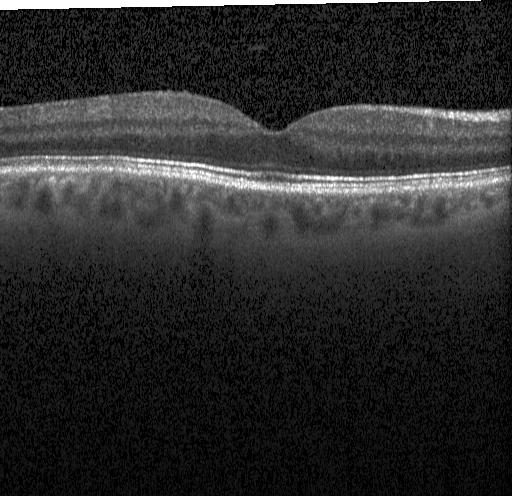

Horizontal scan through the fovea; retinal OCT cross-section.
Dx: no choroidal neovascularization, no diabetic macular edema, and no drusen.